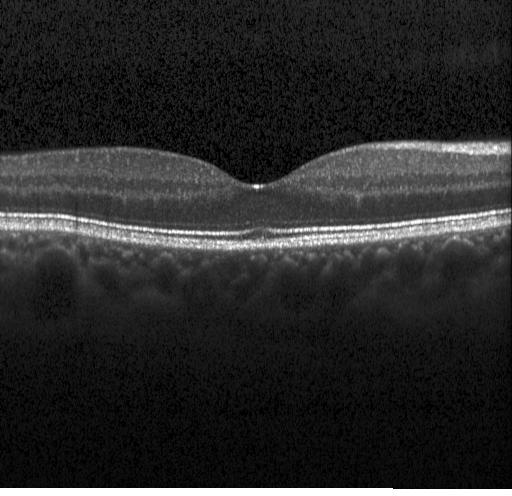
Diagnosis: no choroidal neovascularization, no diabetic macular edema, and no drusen.